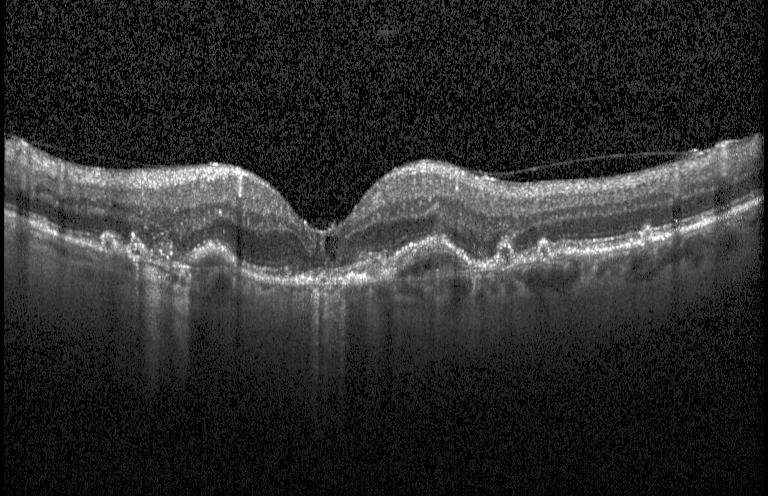
Impression: a choroidal neovascular membrane.